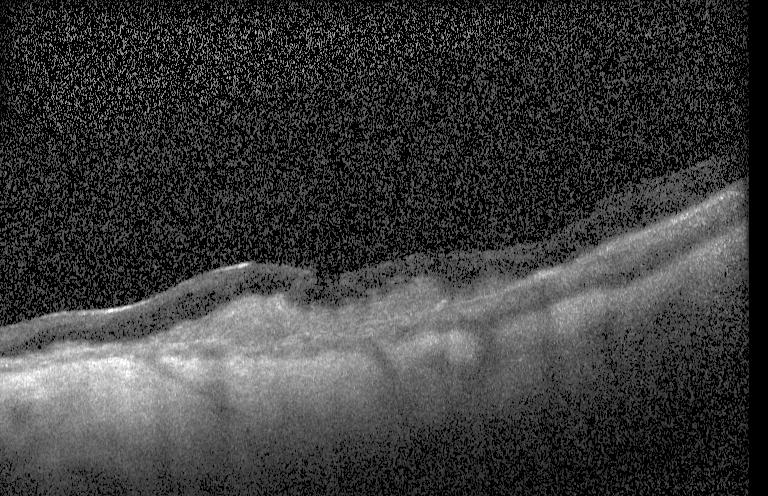
Impression: choroidal neovascularization.